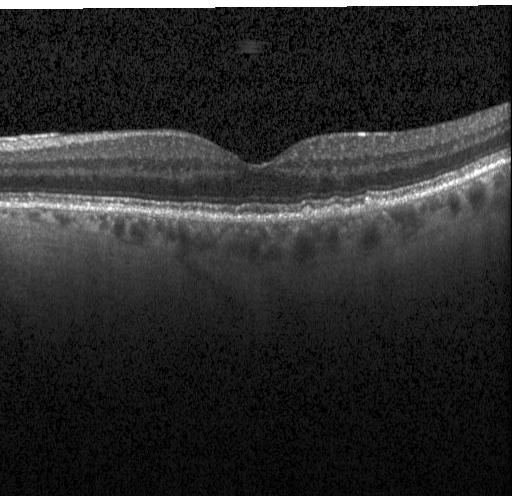

Impression: multiple drusen.